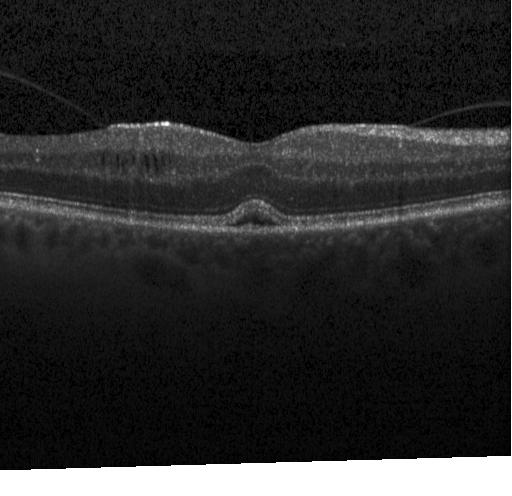
OCT B-scan showing diabetic macular edema (DME).